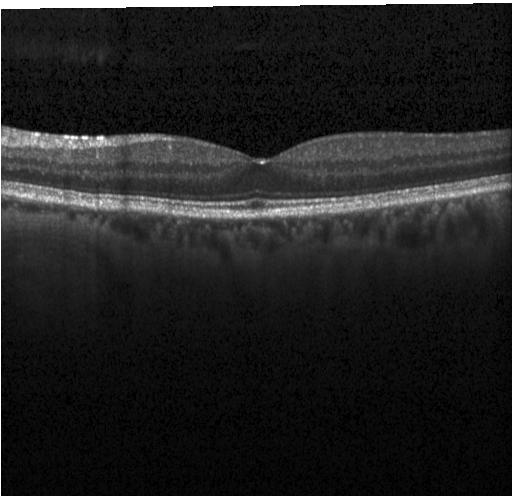
OCT line scan; Heidelberg Spectralis; through the macula.
OCT finding: no choroidal neovascularization, no diabetic macular edema, and no drusen.